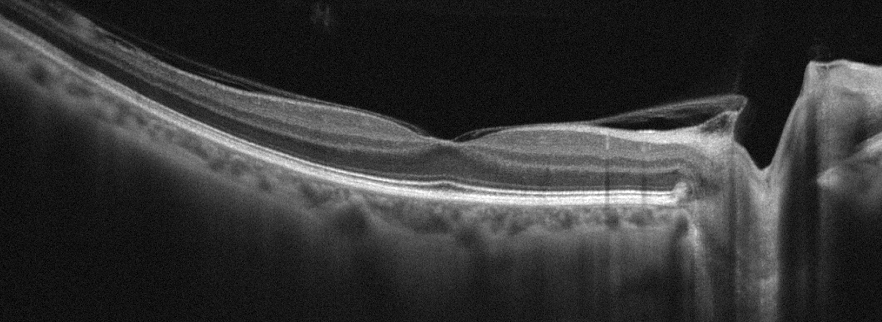 Impression: no evidence of AMD, DME, ERM, RAO, RVO, or VID.